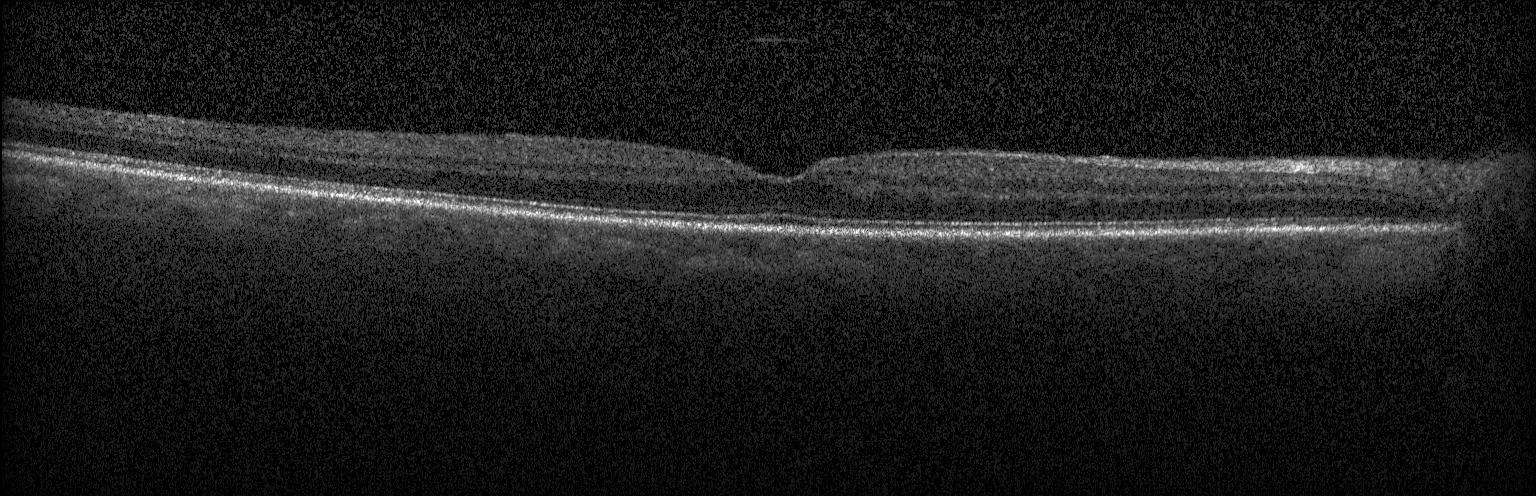
Dx: neither choroidal neovascularization, diabetic macular edema, nor drusen.